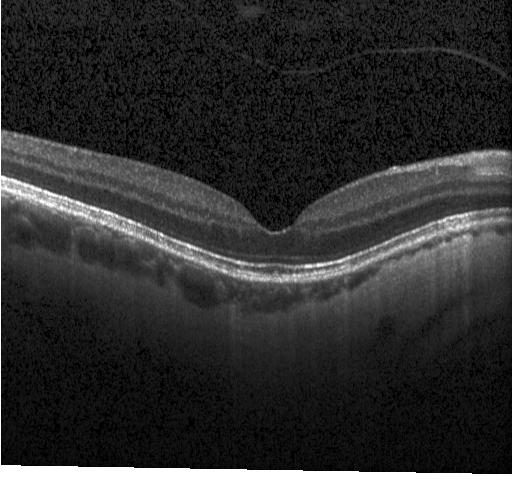 OCT line scan · fovea-centered · acquired on a Heidelberg Spectralis. The scan shows no CNV, no DME, and no drusen.